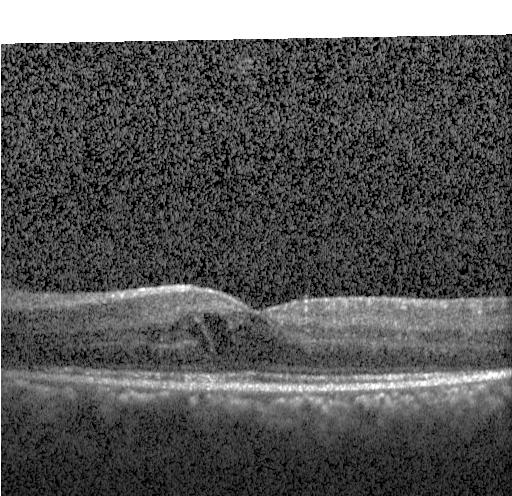

Retinal OCT B-scan — Diabetic macular edema.